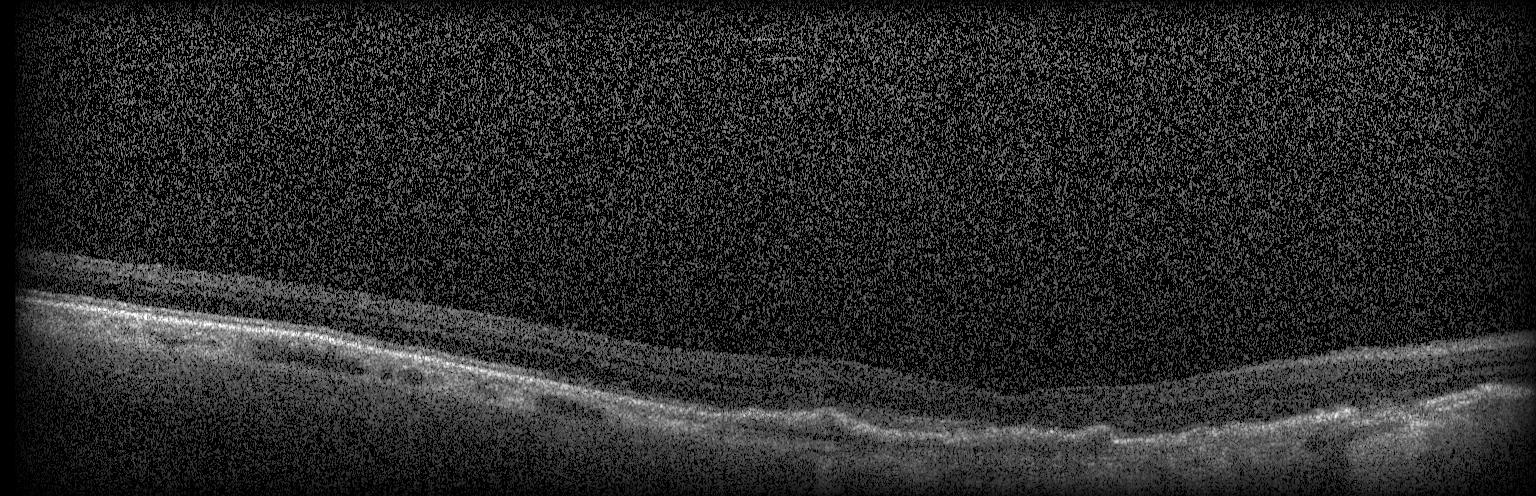

Optical coherence tomography B-scan · horizontal scan through the fovea. Assessment: a choroidal neovascular membrane.